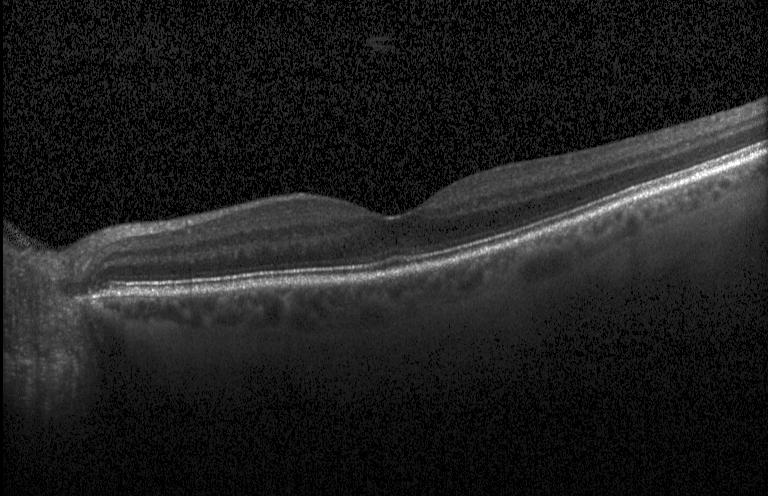 Optical coherence tomography scan. Spectral-domain optical coherence tomography. Acquired on a Heidelberg Spectralis. Centered on the fovea.
Finding: no choroidal neovascularization, diabetic macular edema, or drusen.